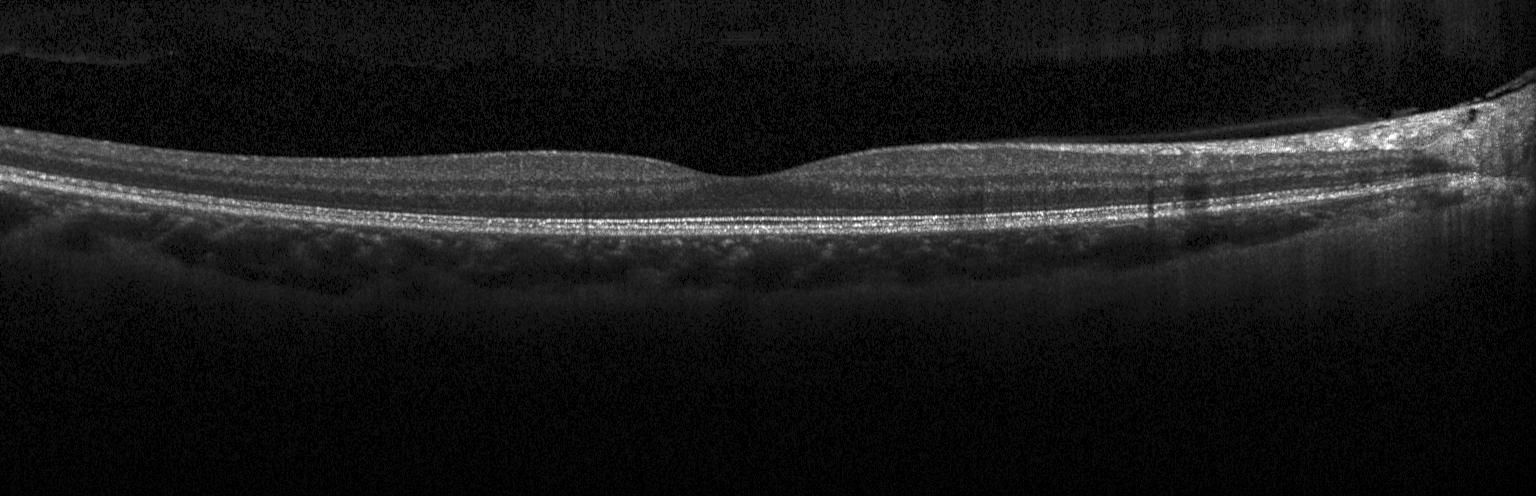 Centered on the fovea; optical coherence tomography B-scan; SD-OCT
Impression: no choroidal neovascularization, diabetic macular edema, or drusen.